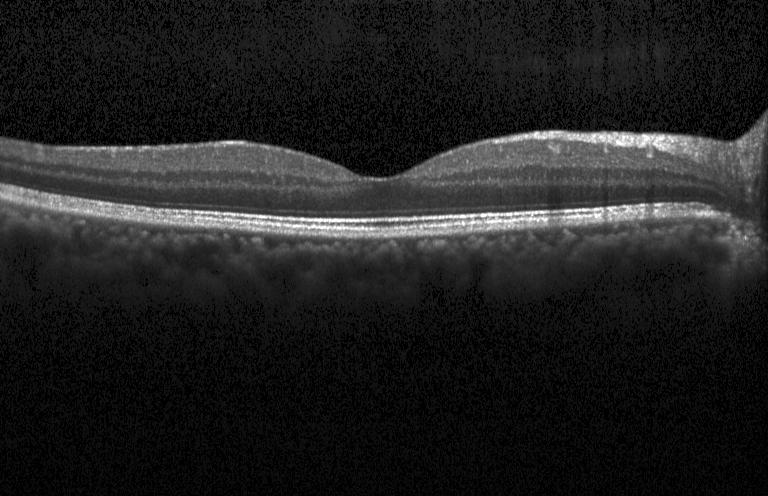

Diagnosis: neither CNV, DME, nor drusen.